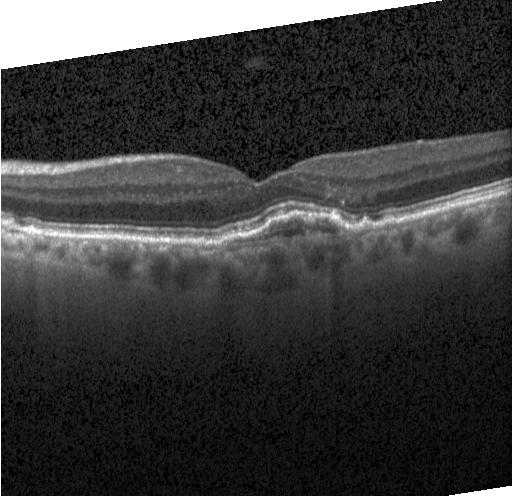
Macular OCT: a choroidal neovascular membrane.